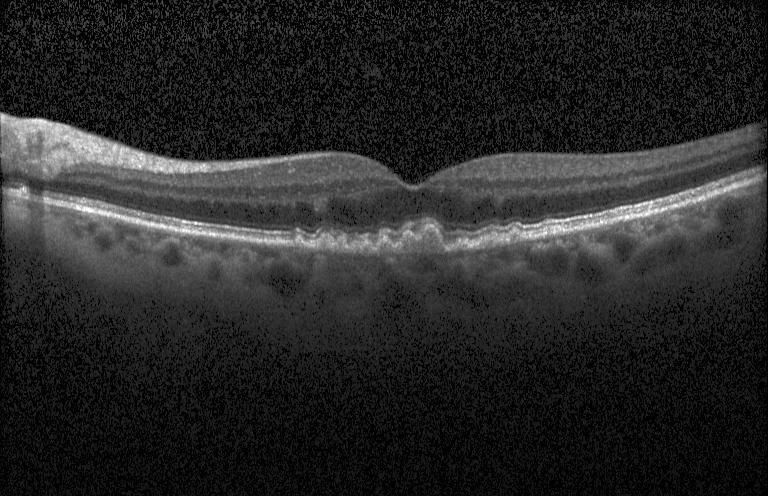

Impression: sub-RPE drusenoid deposits.